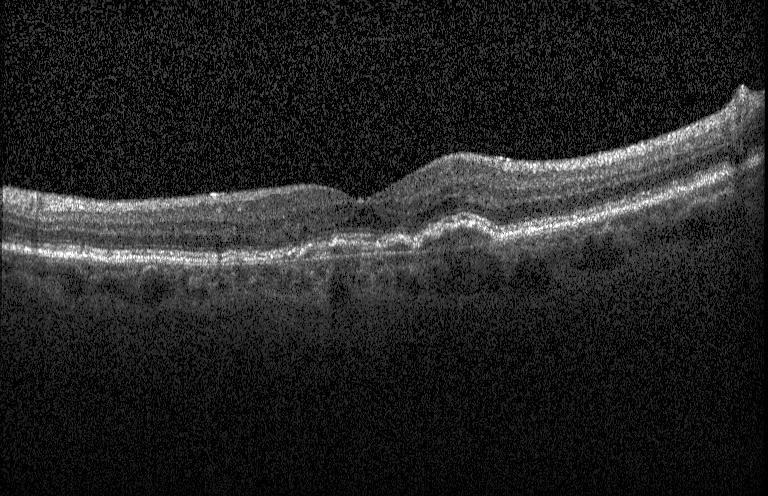 Retinal OCT cross-section, horizontal scan through the fovea, SD-OCT. A choroidal neovascular membrane.